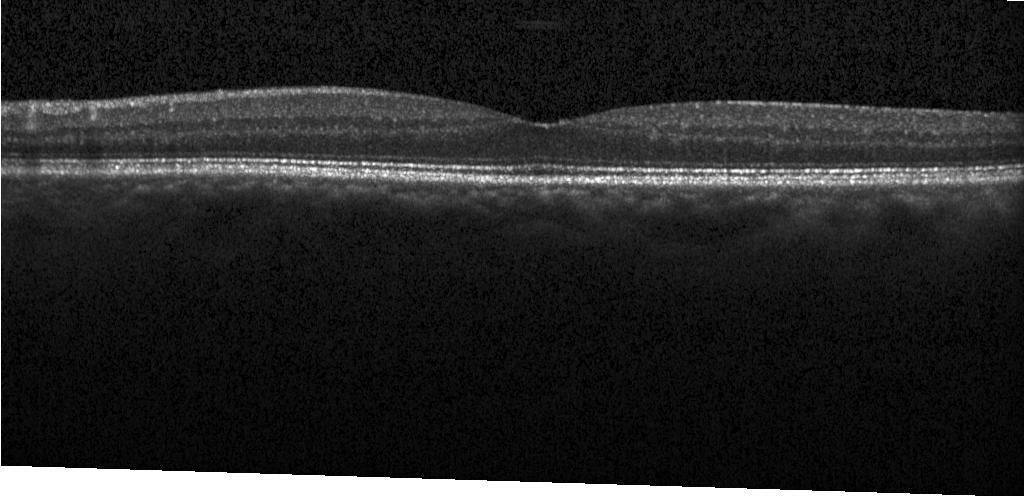 Retinal OCT B-scan. Horizontal scan through the fovea. No CNV, DME, or drusen.